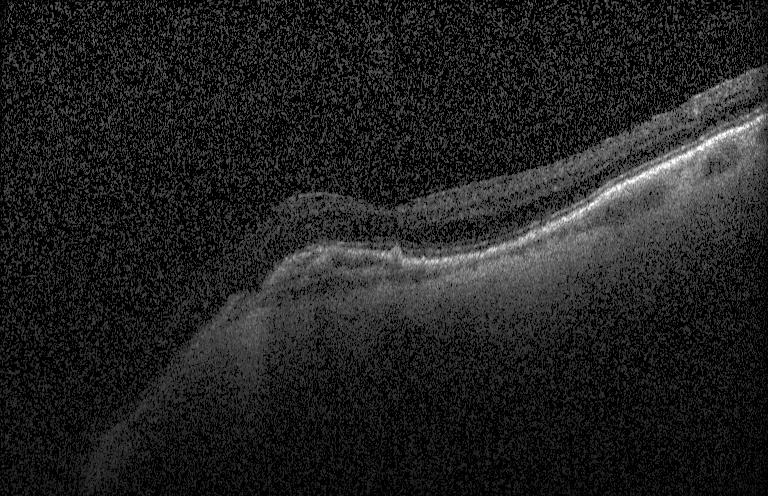
OCT finding: a choroidal neovascular membrane.